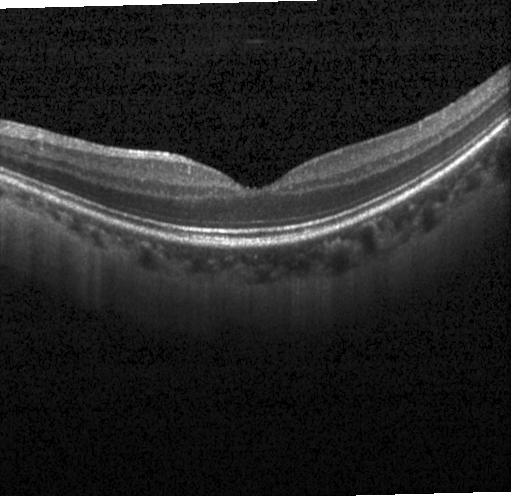 Heidelberg Spectralis; OCT B-scan; centered on the fovea. Finding: no choroidal neovascularization, no diabetic macular edema, and no drusen.